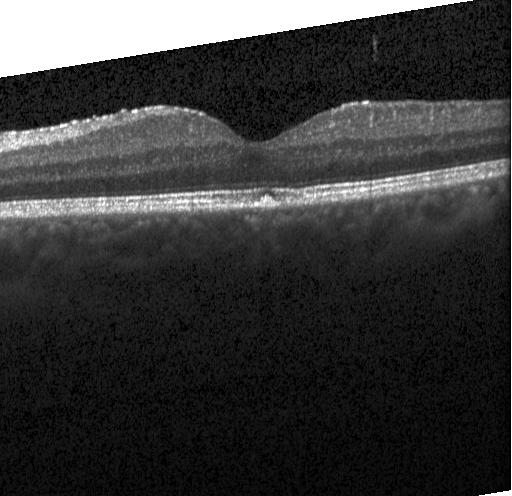
OCT B-scan showing sub-RPE drusenoid deposits.